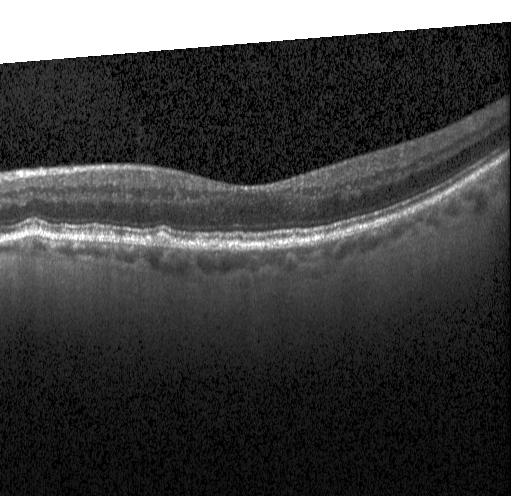 Retinal OCT B-scan.
Drusen.